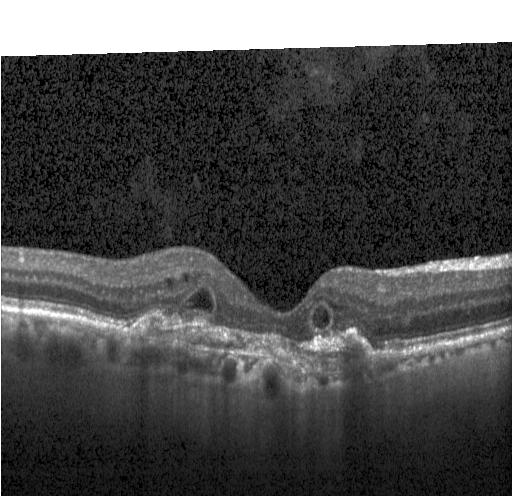
Optical coherence tomography scan — Assessment: a choroidal neovascular membrane.